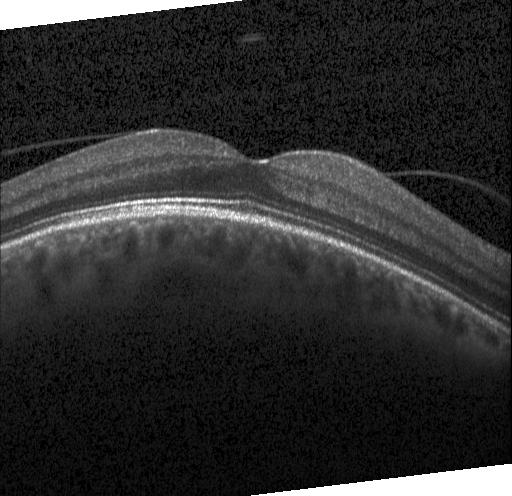 Centered on the fovea; Heidelberg Spectralis OCT system; retinal OCT cross-section; spectral-domain OCT
Diagnosis: no evidence of choroidal neovascularization, diabetic macular edema, or drusen.